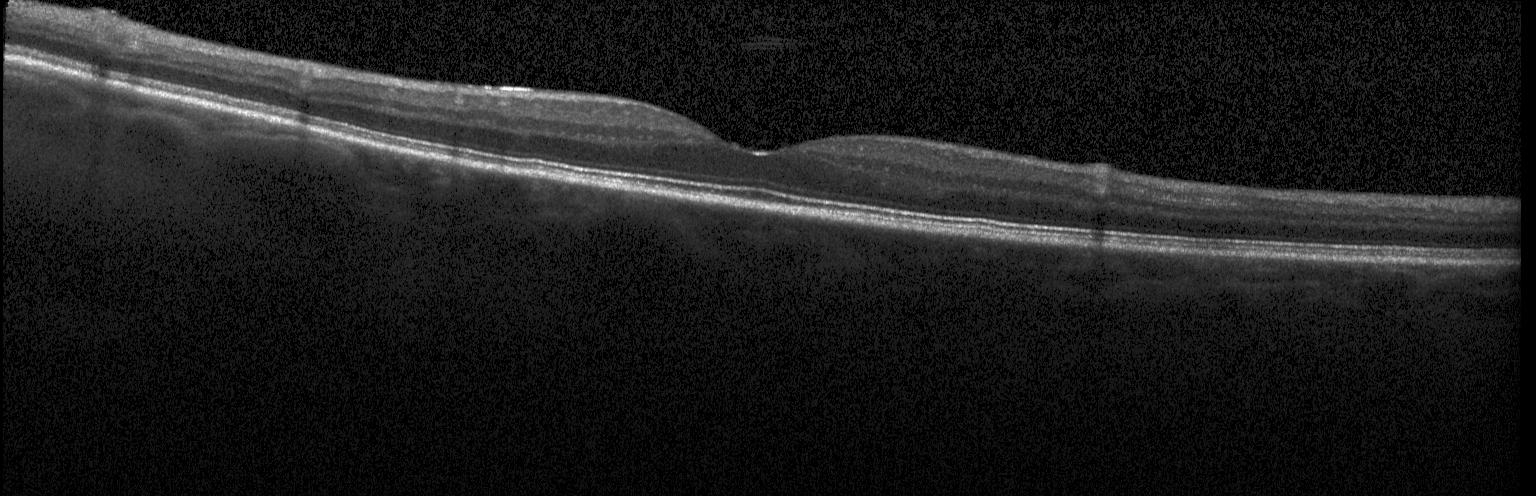

Instrument: Heidelberg Spectralis · OCT B-scan. Finding: no evidence of CNV, DME, or drusen.